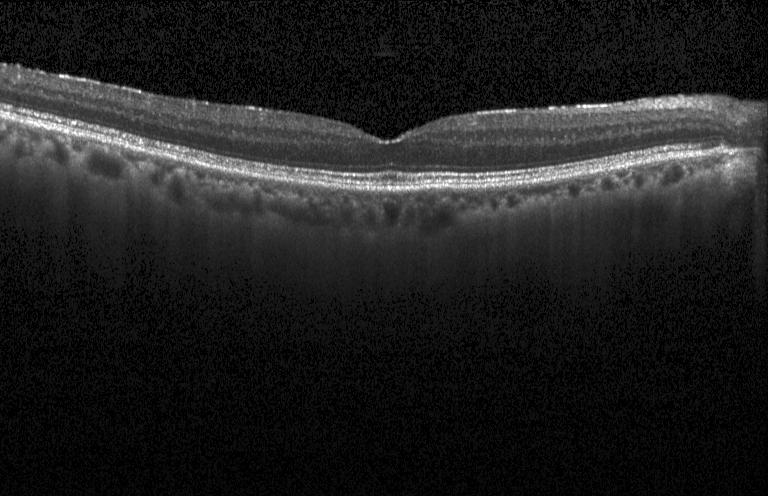
The scan shows neither choroidal neovascularization, diabetic macular edema, nor drusen.